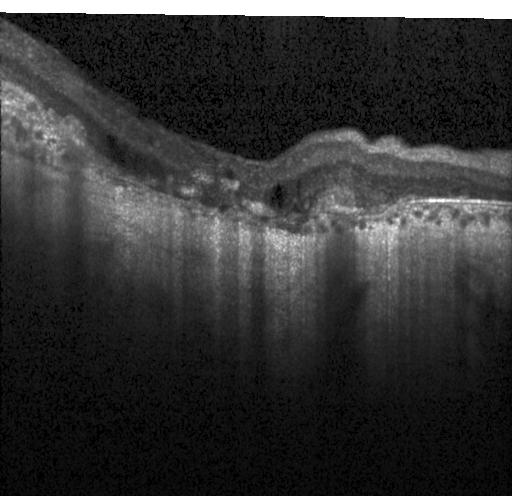
Retinal OCT B-scan · spectral-domain optical coherence tomography · fovea-centered. Impression: a choroidal neovascular membrane.